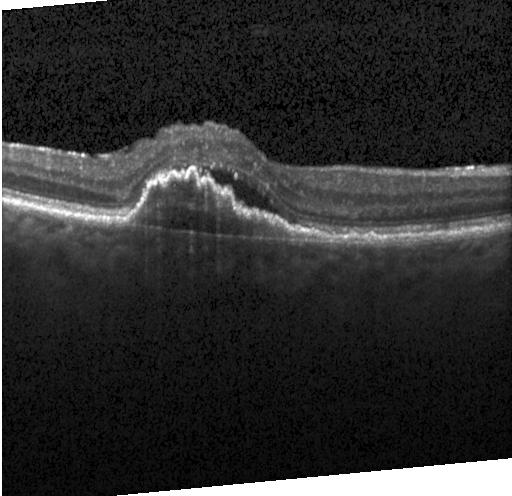 Optical coherence tomography scan
Finding: CNV.